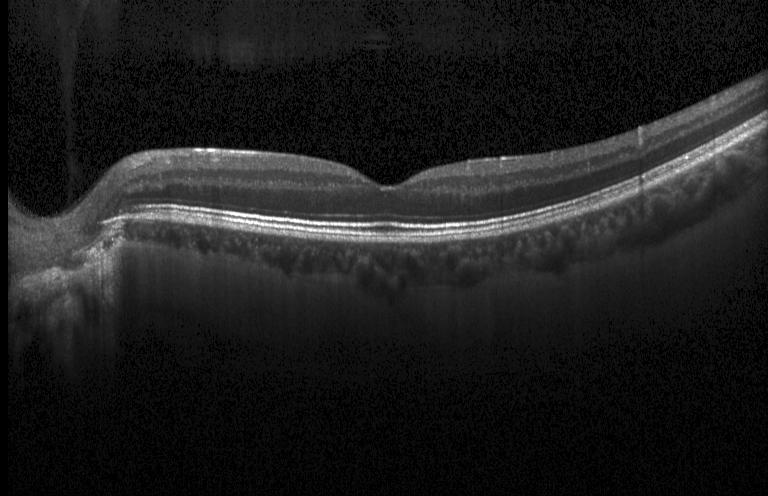
Acquired on a Heidelberg Spectralis. SD-OCT. Retinal OCT B-scan
OCT finding: no CNV, DME, or drusen.